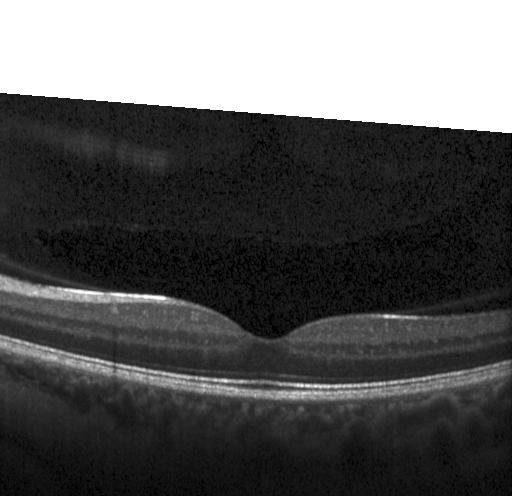
The scan shows no CNV, no DME, and no drusen.